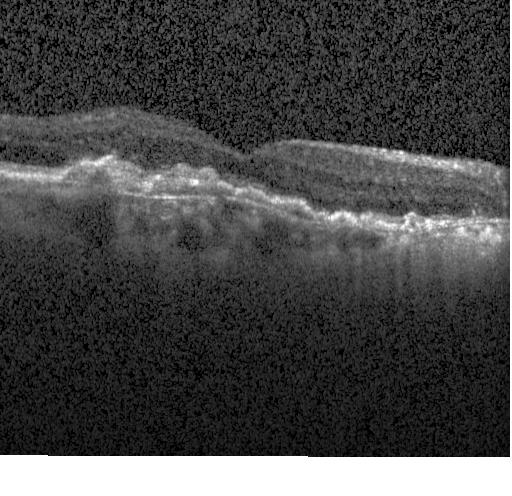 Spectral-domain OCT, instrument: Heidelberg Spectralis, fovea-centered, retinal OCT cross-section.
Impression: a choroidal neovascular membrane.